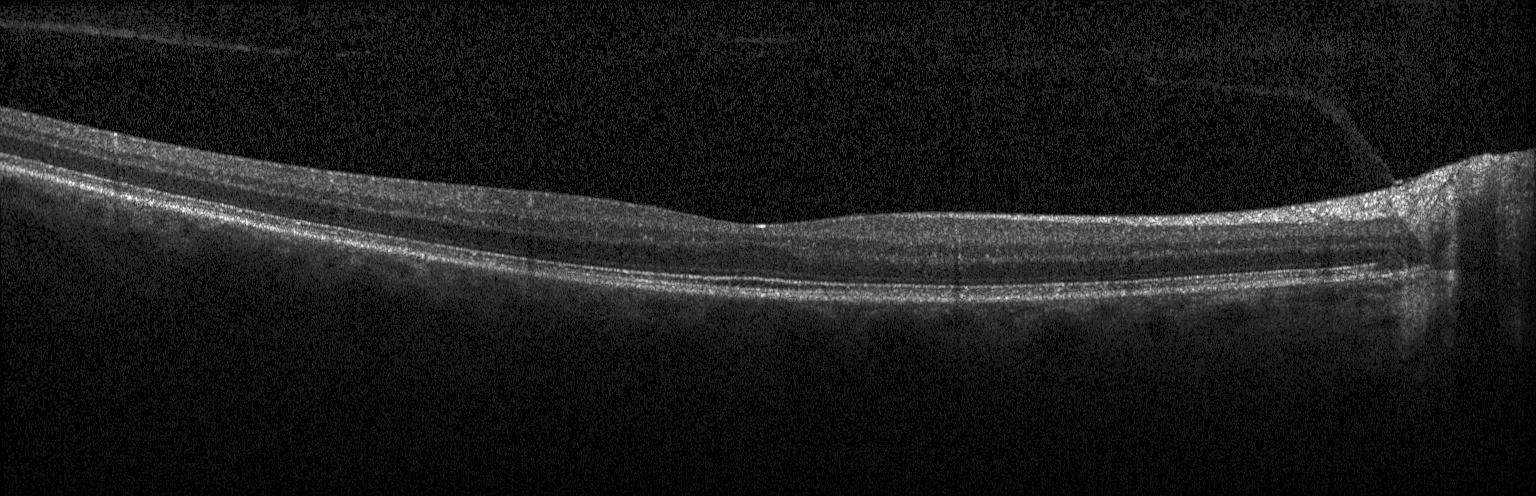
This B-scan demonstrates no evidence of choroidal neovascularization, diabetic macular edema, or drusen.